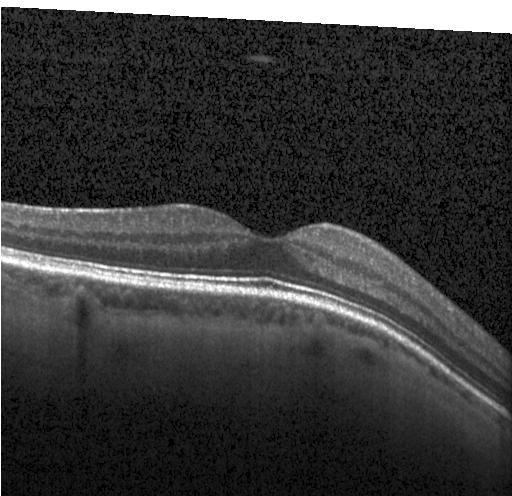
Neither CNV, DME, nor drusen.